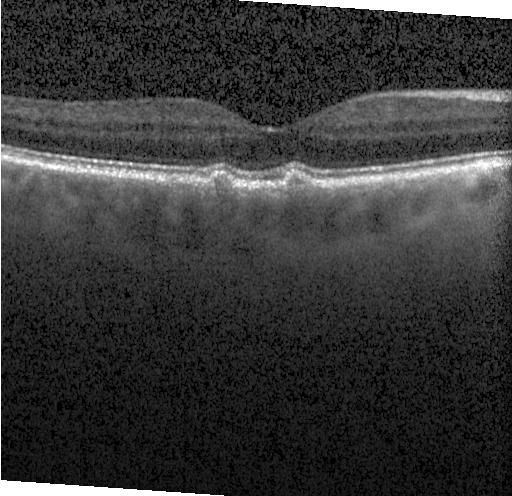 OCT B-scan · through the macula
Diagnosis: sub-RPE drusenoid deposits.